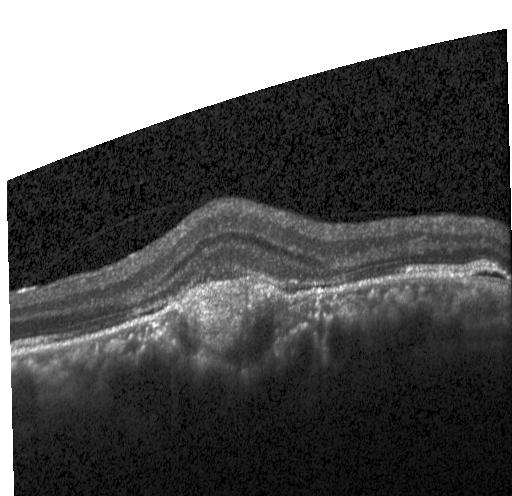 Finding: a choroidal neovascular membrane.